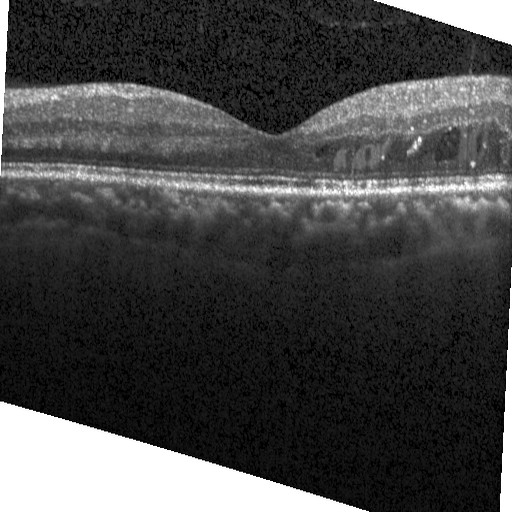 SD-OCT · retinal OCT cross-section — Finding: DME.